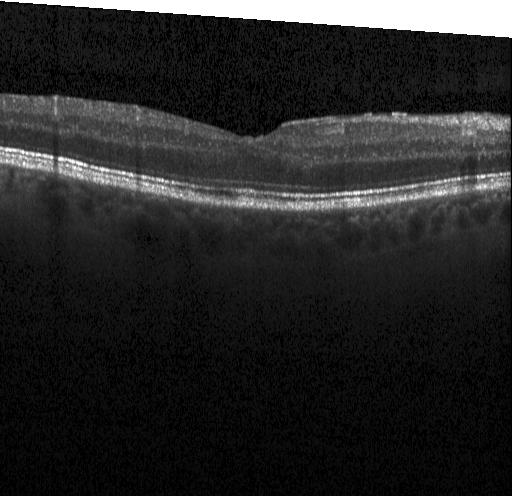

Retinal OCT cross-section showing no choroidal neovascularization, no diabetic macular edema, and no drusen.